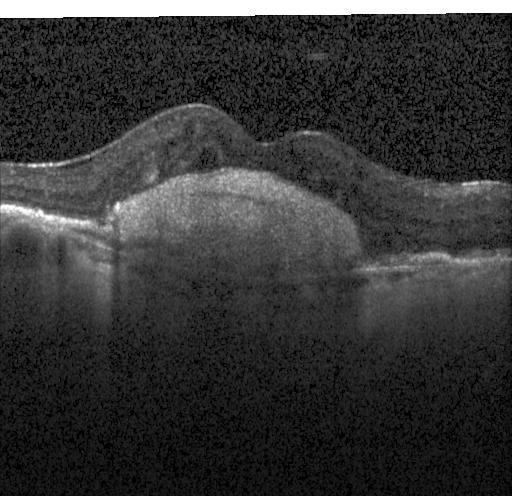
Retinal OCT B-scan. Spectral-domain optical coherence tomography. Horizontal scan through the fovea. Heidelberg Spectralis — The scan shows a choroidal neovascular membrane.